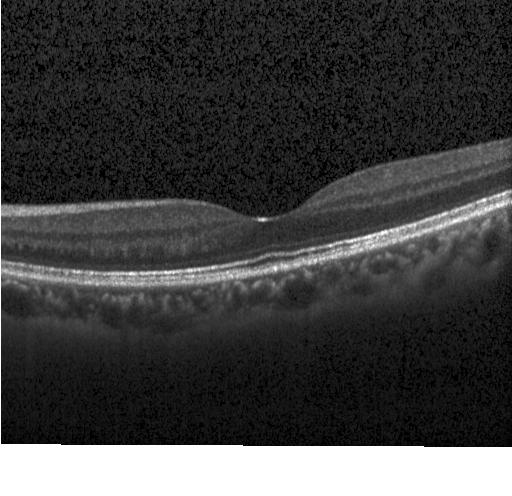

OCT B-scan.
Finding: no choroidal neovascularization, no diabetic macular edema, and no drusen.